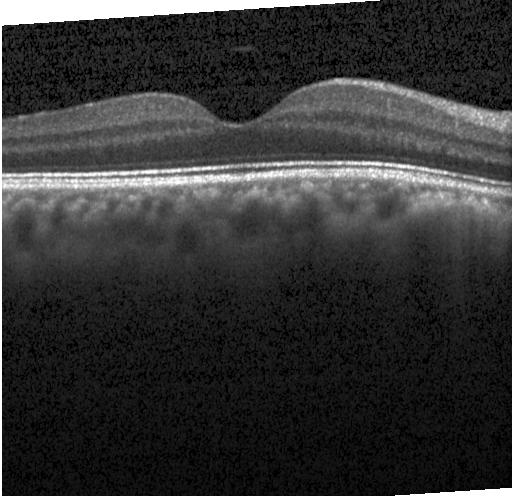

SD-OCT; optical coherence tomography scan; Heidelberg Spectralis OCT system; centered on the fovea.
Finding: no choroidal neovascularization, diabetic macular edema, or drusen.